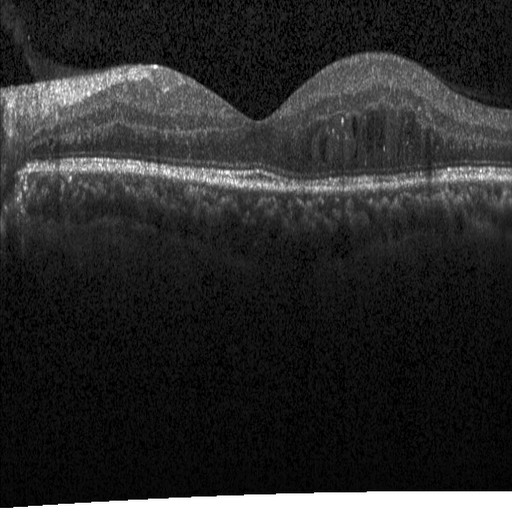 OCT B-scan. Dx: DME.